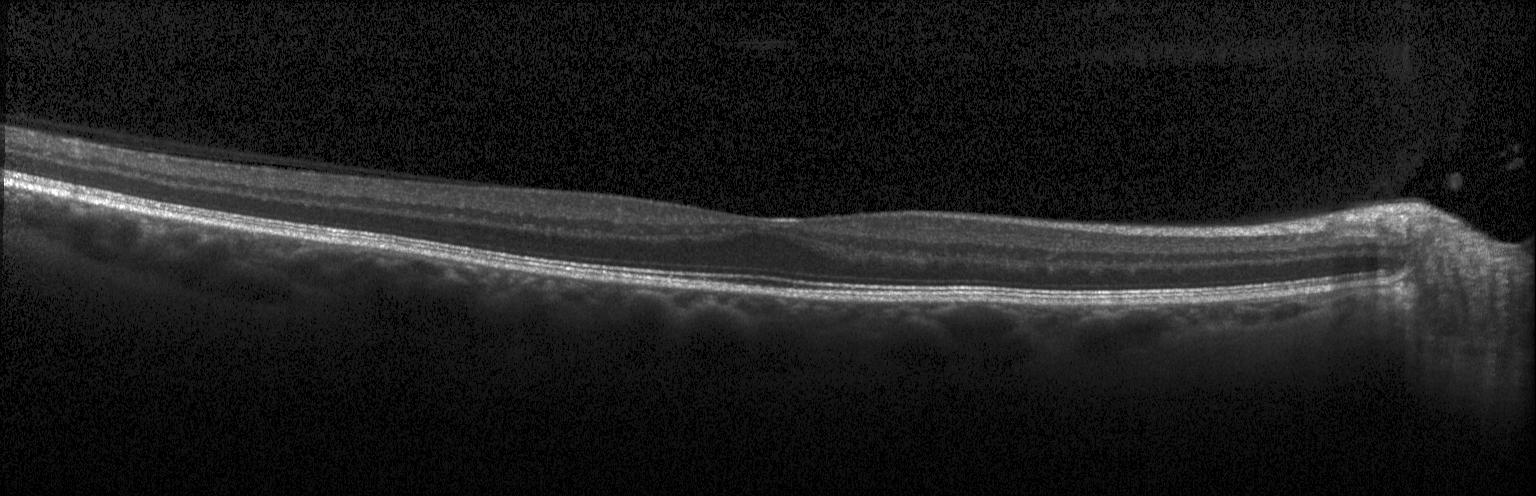
Retinal OCT B-scan. Diagnosis: neither choroidal neovascularization, diabetic macular edema, nor drusen.